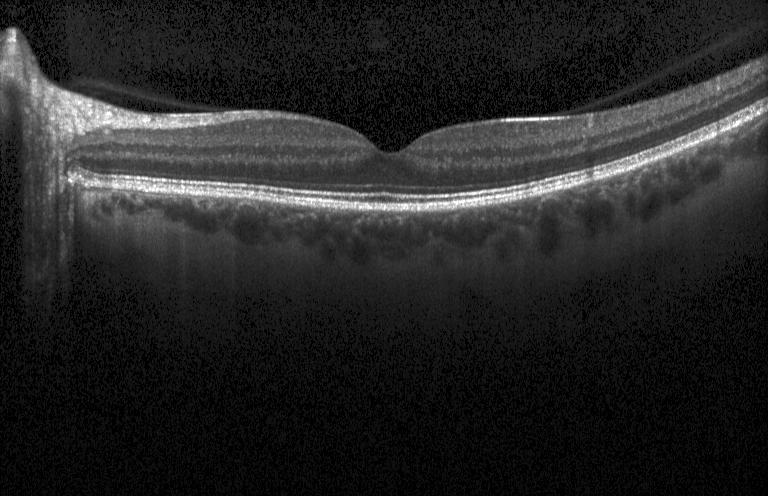 Diagnosis: no evidence of choroidal neovascularization, diabetic macular edema, or drusen.